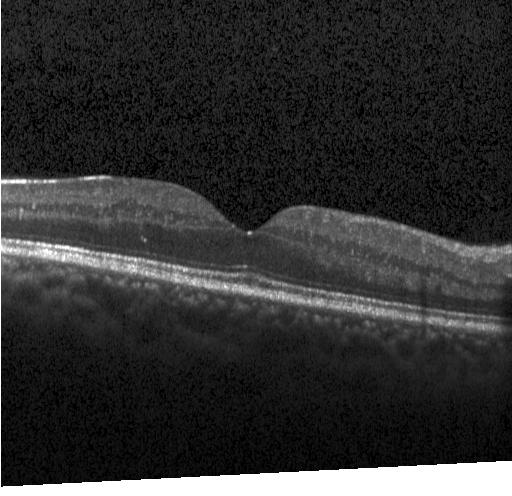
OCT B-scan — No evidence of choroidal neovascularization, diabetic macular edema, or drusen.